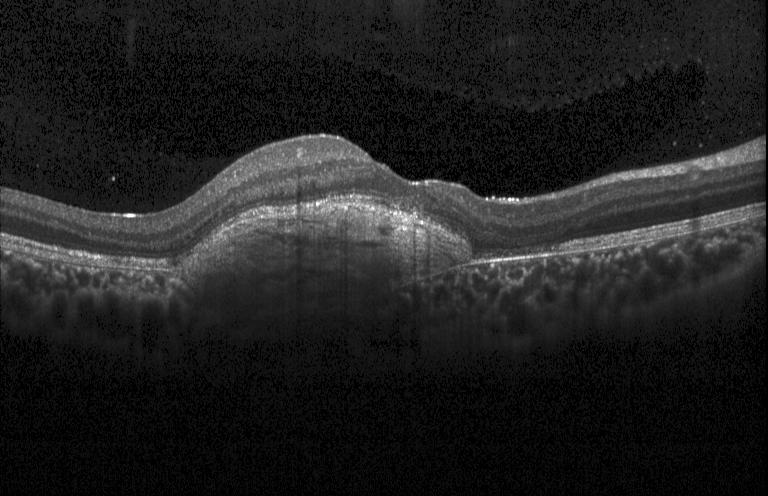 Optical coherence tomography scan. Macular scan. Heidelberg Spectralis OCT system.
The scan shows choroidal neovascularization.